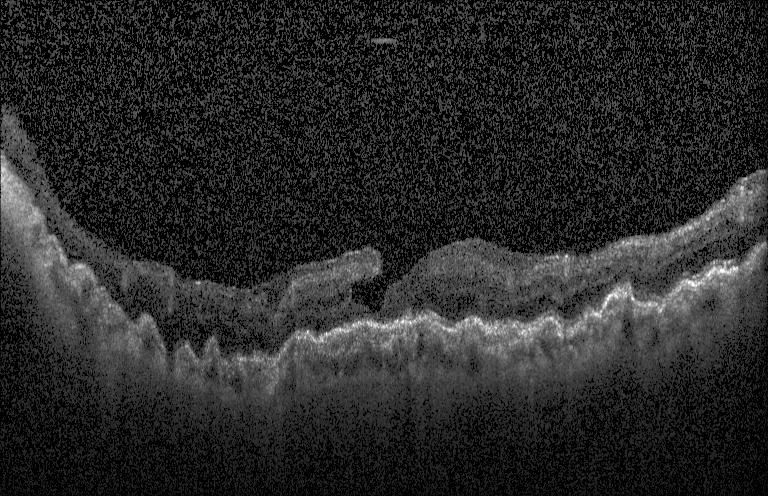

Instrument: Heidelberg Spectralis · fovea-centered · retinal OCT B-scan.
Impression: choroidal neovascularization.